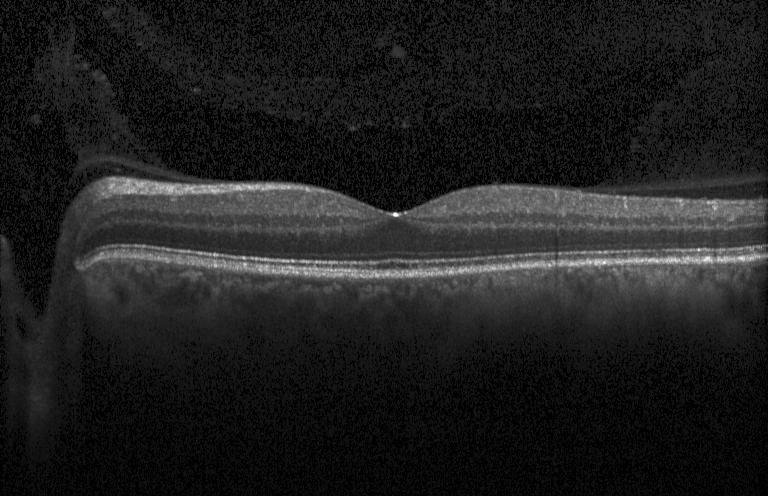

OCT line scan; Heidelberg Spectralis OCT system; spectral-domain optical coherence tomography; fovea-centered
Assessment: no CNV, DME, or drusen.